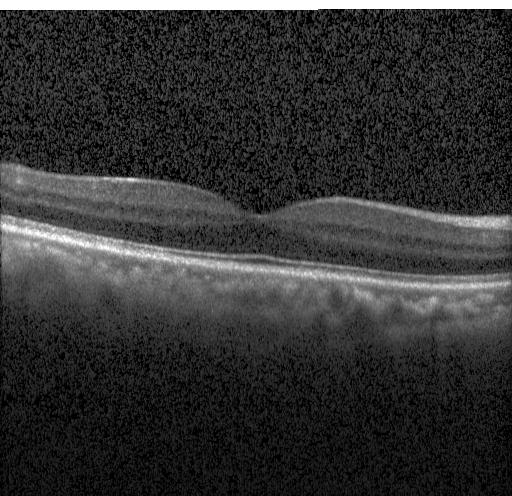 The scan shows no evidence of CNV, DME, or drusen.